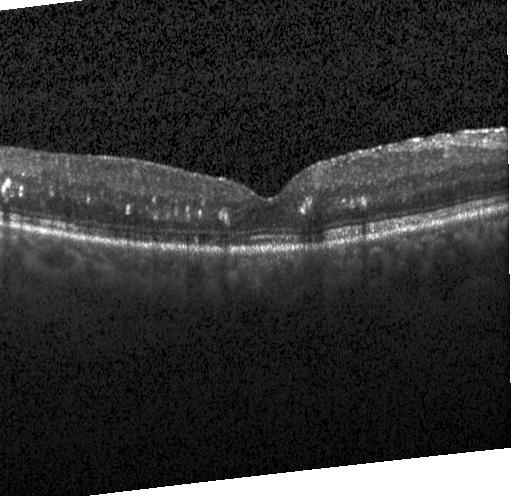

Diagnosis: diabetic macular edema.